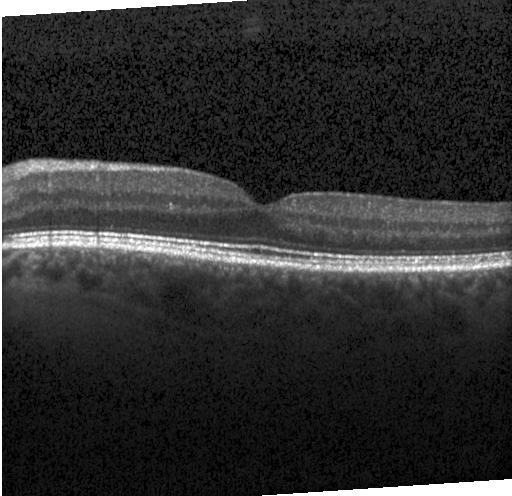 Macular OCT: no choroidal neovascularization, diabetic macular edema, or drusen.